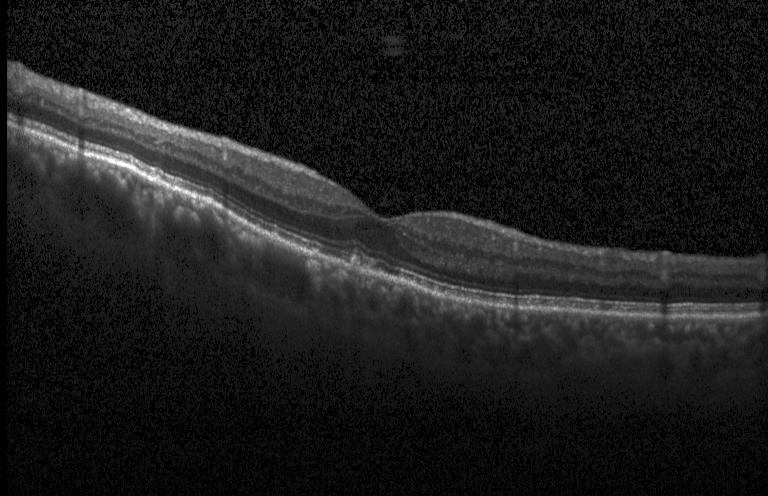
Spectral-domain optical coherence tomography, retinal OCT B-scan, Heidelberg Spectralis OCT system, fovea-centered.
Macular OCT: multiple drusen.